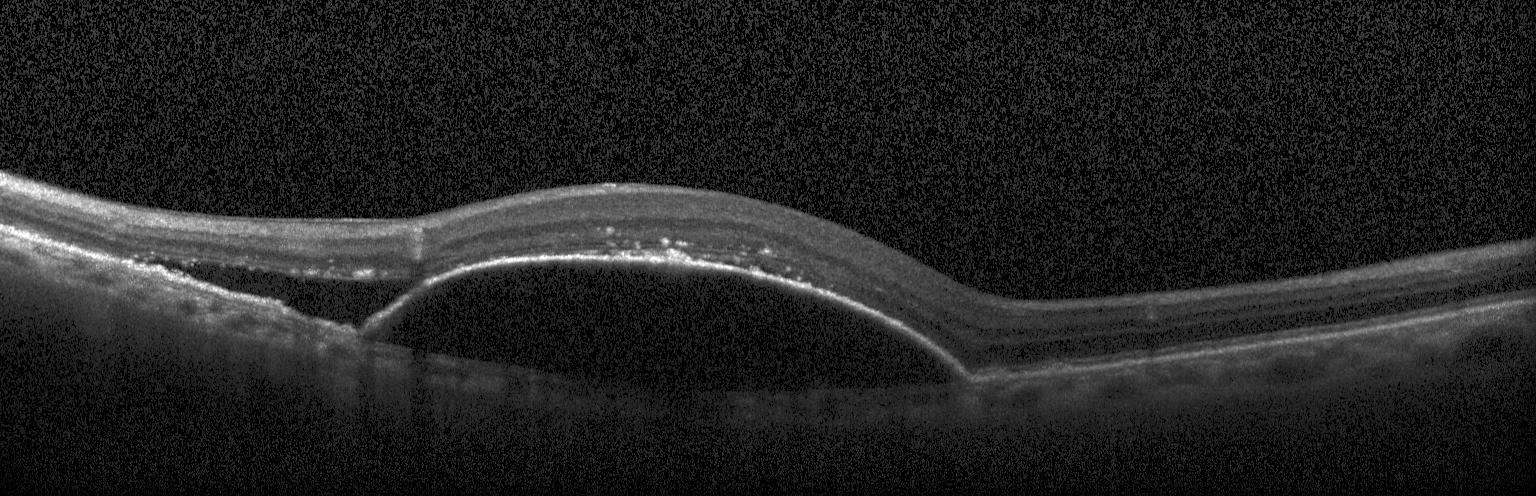

Optical coherence tomography B-scan. Diagnosis: CNV.